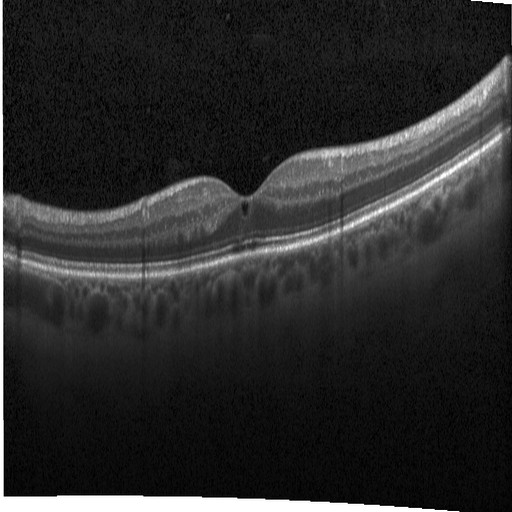
Finding: diabetic macular edema (DME).